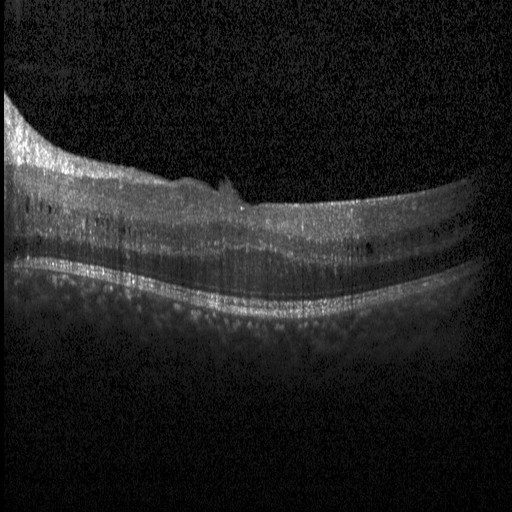

Assessment: DME.